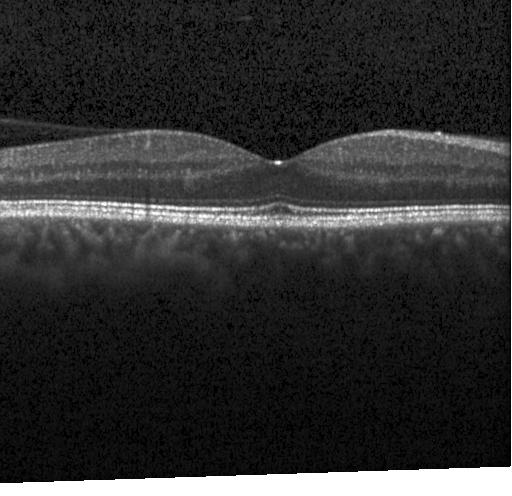
OCT B-scan showing neither CNV, DME, nor drusen.